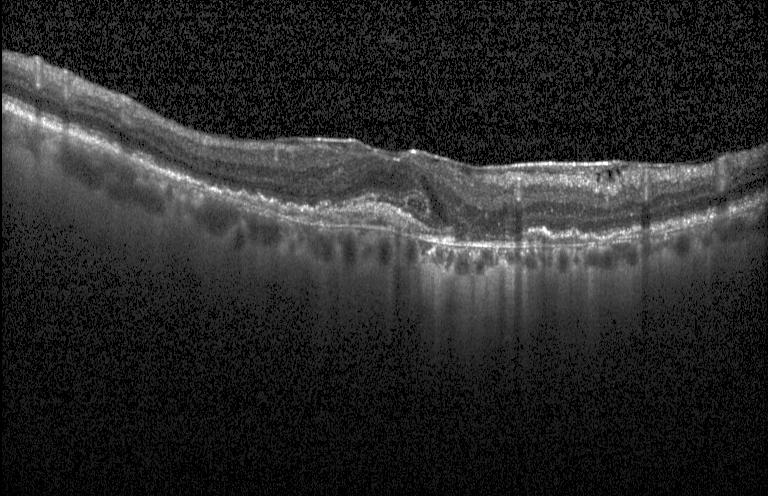
SD-OCT · optical coherence tomography scan · centered on the fovea. Impression: choroidal neovascularization.